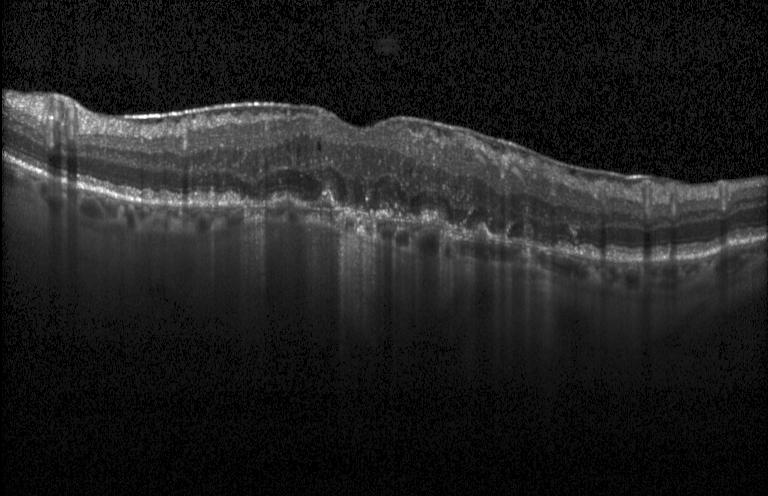
Macular scan, Heidelberg Spectralis OCT system, retinal OCT B-scan. Assessment: a choroidal neovascular membrane.